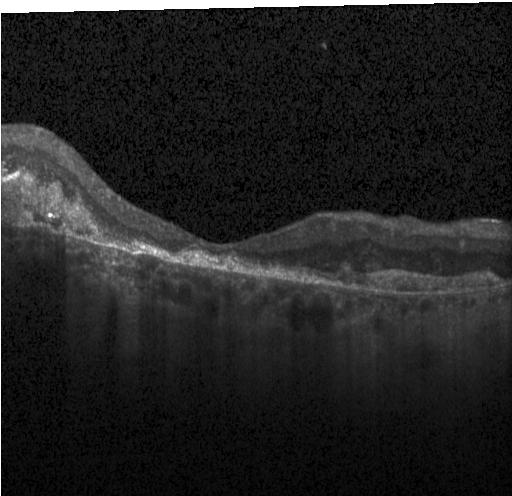
Optical coherence tomography B-scan — Diagnosis: choroidal neovascularization (CNV).